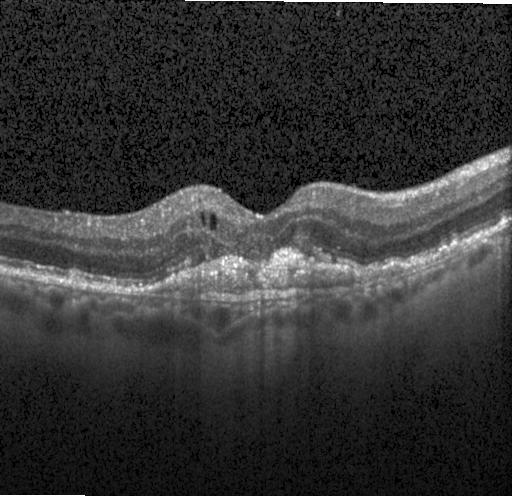
Acquired on a Heidelberg Spectralis · SD-OCT · retinal OCT cross-section
Finding: a choroidal neovascular membrane.